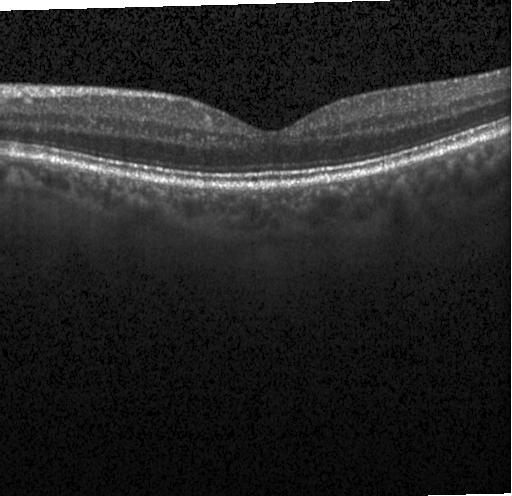 Retinal OCT B-scan. SD-OCT. Heidelberg Spectralis OCT system
This B-scan demonstrates no choroidal neovascularization, no diabetic macular edema, and no drusen.